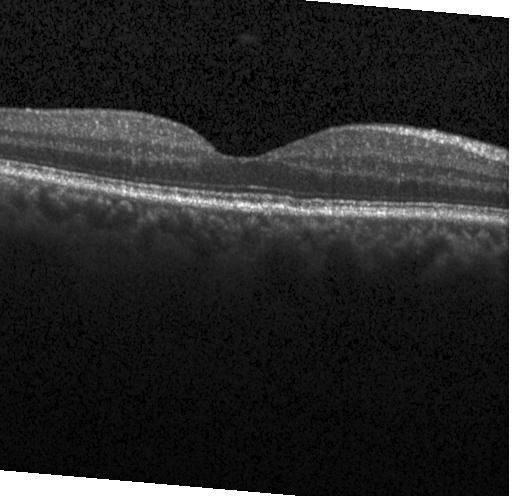 OCT finding: no CNV, no DME, and no drusen.